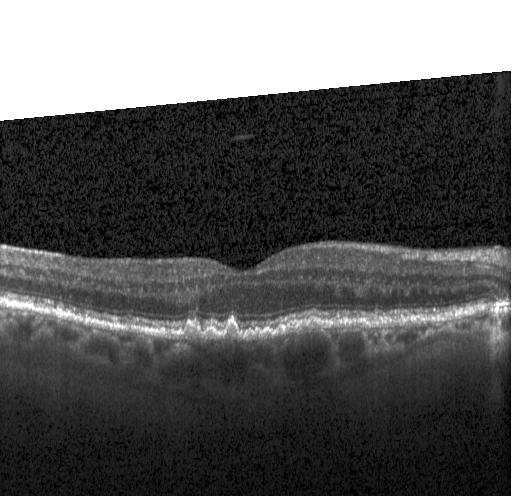
Retinal OCT B-scan.
Diagnosis: drusen.